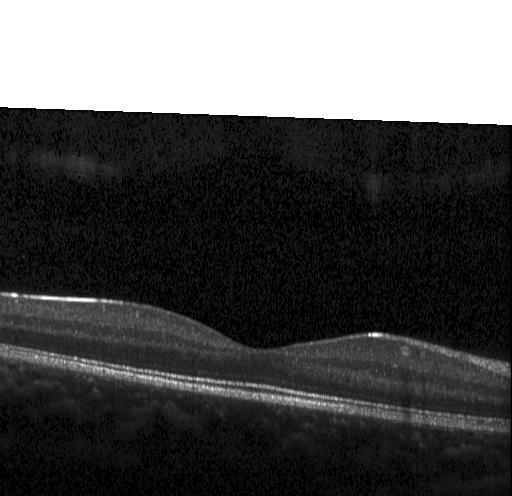 Heidelberg Spectralis OCT system. OCT B-scan. Diagnosis: neither CNV, DME, nor drusen.